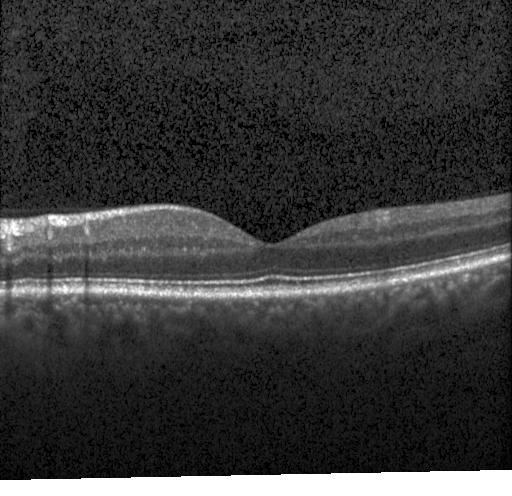
Spectral-domain optical coherence tomography · optical coherence tomography scan · Heidelberg Spectralis OCT system · fovea-centered. Impression: no evidence of choroidal neovascularization, diabetic macular edema, or drusen.